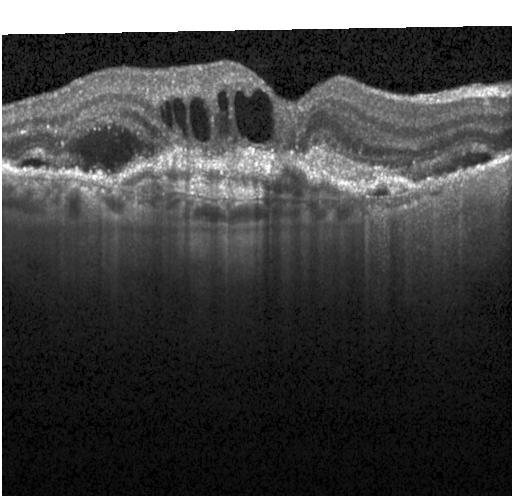
Dx: a choroidal neovascular membrane.